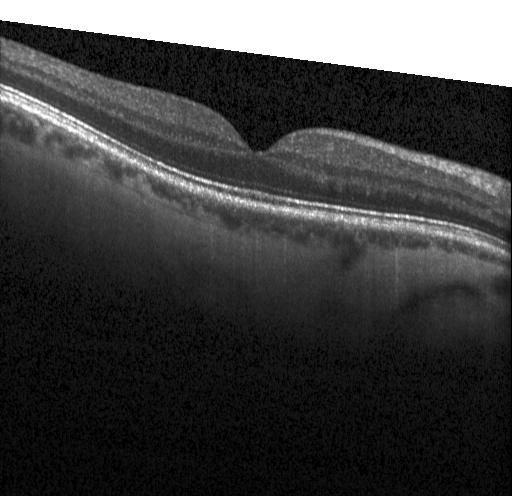 Spectral-domain optical coherence tomography. OCT line scan.
Diagnosis: no evidence of choroidal neovascularization, diabetic macular edema, or drusen.